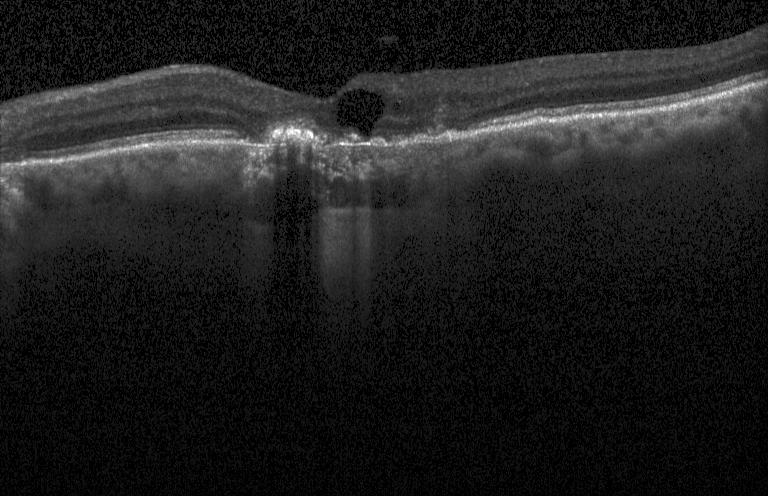
Instrument: Heidelberg Spectralis. Spectral-domain OCT. Optical coherence tomography B-scan. Impression: a choroidal neovascular membrane.